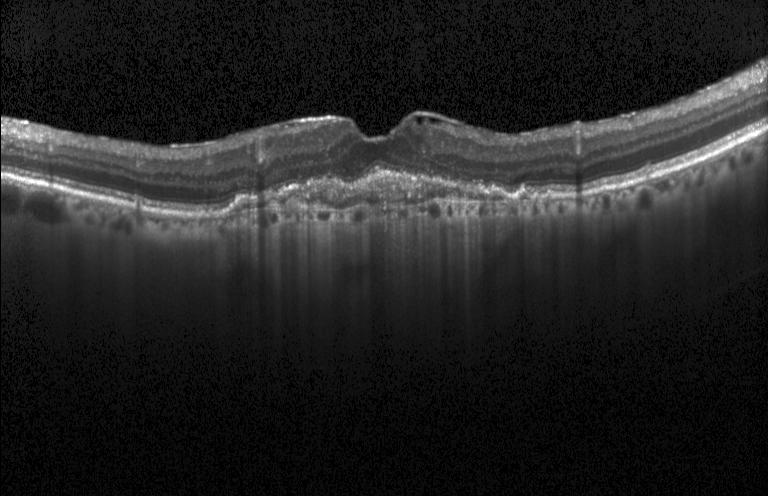
Optical coherence tomography B-scan. Finding: a choroidal neovascular membrane.